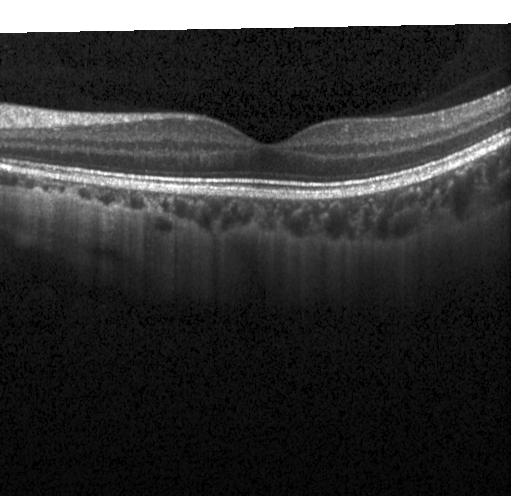

Optical coherence tomography scan — Dx: no evidence of choroidal neovascularization, diabetic macular edema, or drusen.